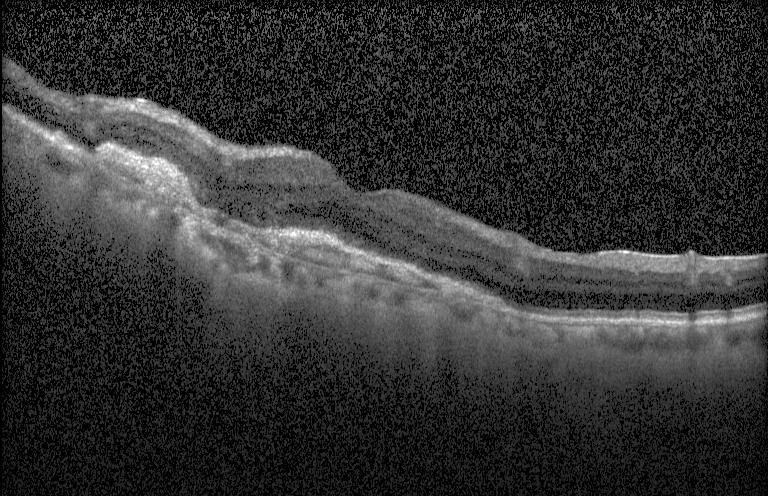
Spectral-domain optical coherence tomography; optical coherence tomography scan; through the macula; Heidelberg Spectralis. OCT finding: choroidal neovascularization.